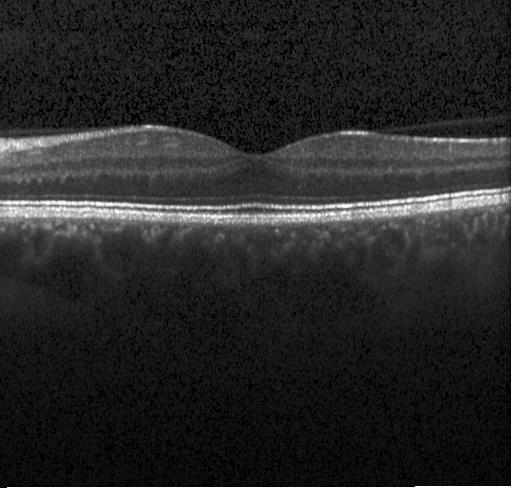
Instrument: Heidelberg Spectralis · optical coherence tomography scan. Impression: neither choroidal neovascularization, diabetic macular edema, nor drusen.